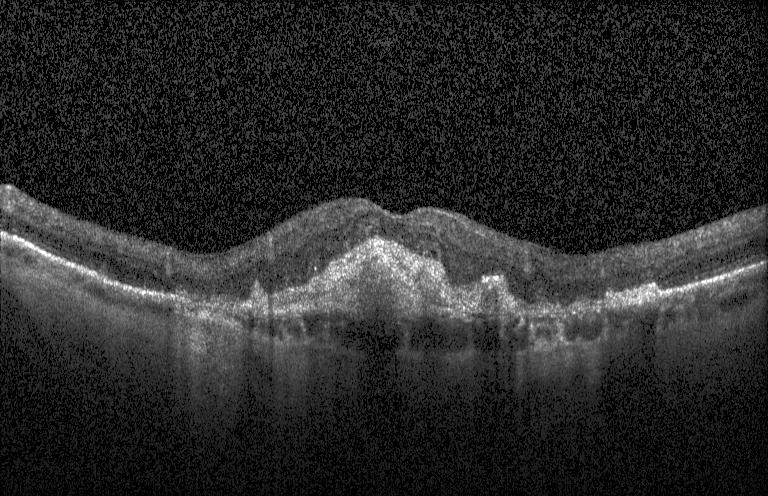

OCT B-scan showing choroidal neovascularization (CNV).